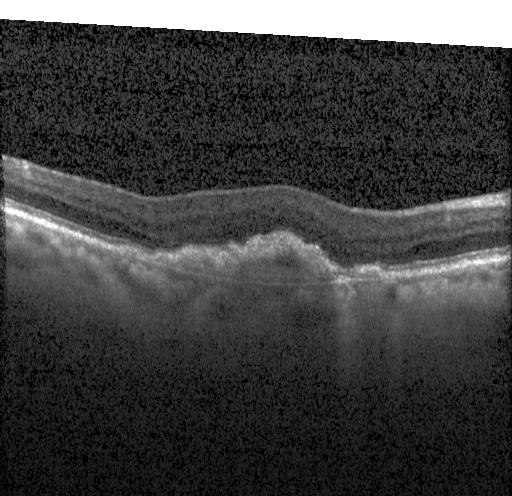
Optical coherence tomography B-scan. OCT finding: a choroidal neovascular membrane.